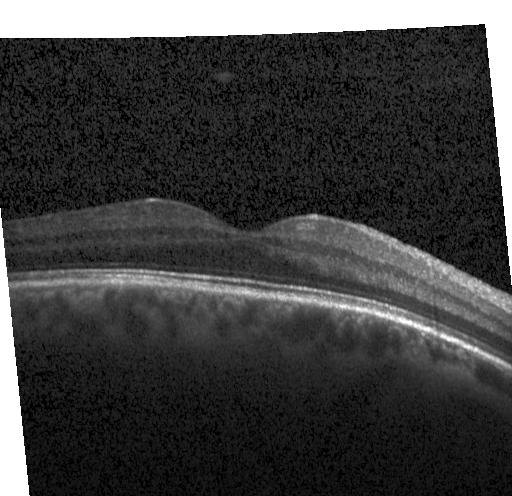
Retinal OCT cross-section.
Diagnosis: neither CNV, DME, nor drusen.